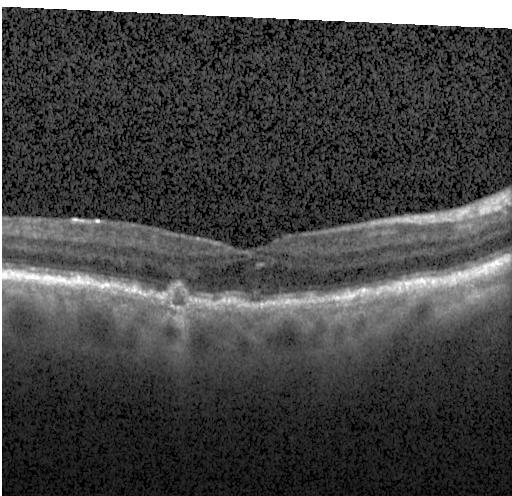
Retinal OCT cross-section showing sub-RPE drusenoid deposits.